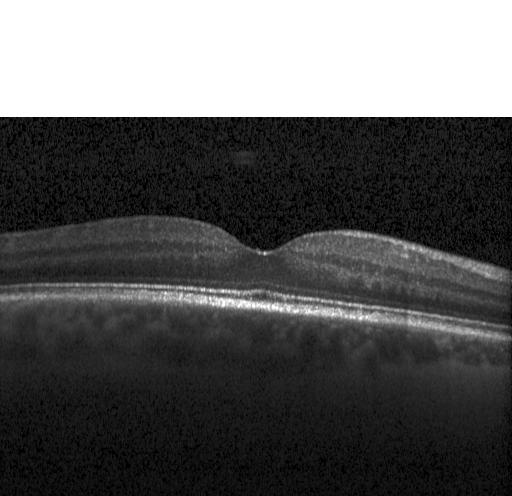
Impression: no CNV, no DME, and no drusen.